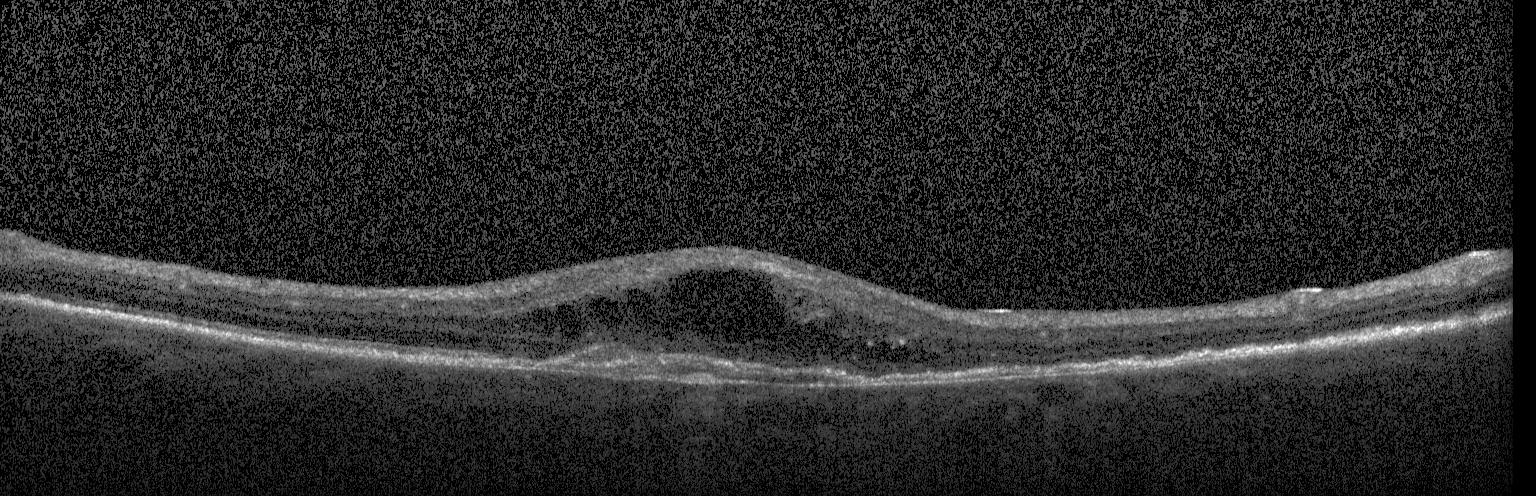

Optical coherence tomography scan, Heidelberg Spectralis OCT system
Diagnosis: choroidal neovascularization (CNV).